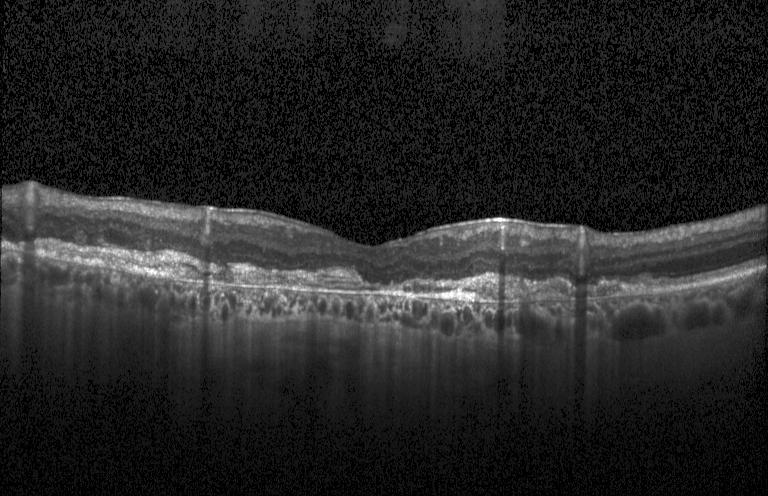

Horizontal scan through the fovea; Heidelberg Spectralis OCT system; retinal OCT cross-section; spectral-domain OCT
This B-scan demonstrates choroidal neovascularization.